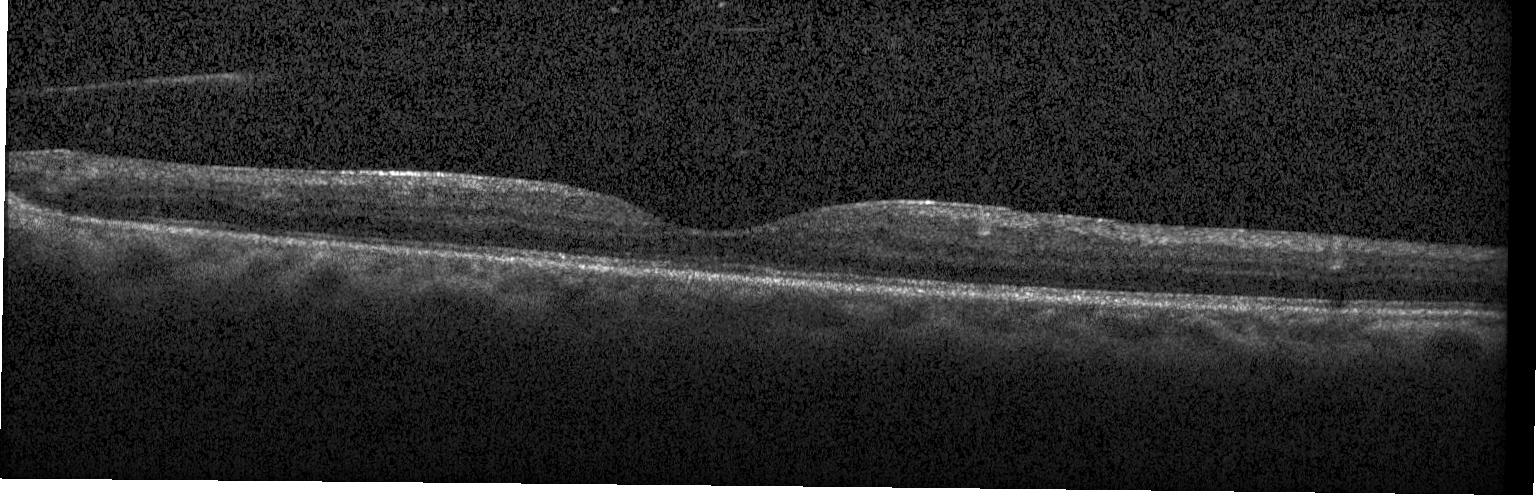
OCT B-scan.
The scan shows no choroidal neovascularization, diabetic macular edema, or drusen.